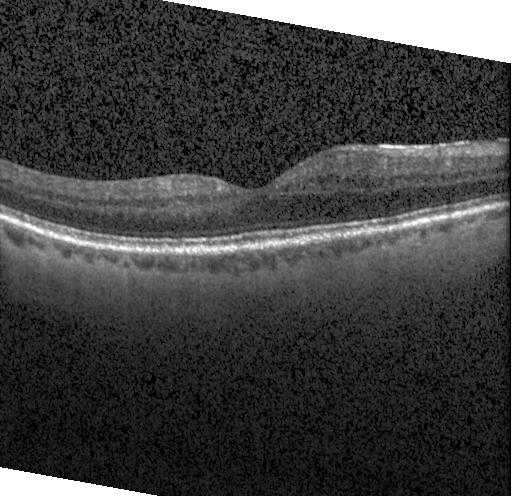

Horizontal scan through the fovea. Optical coherence tomography scan. Instrument: Heidelberg Spectralis — No evidence of choroidal neovascularization, diabetic macular edema, or drusen.